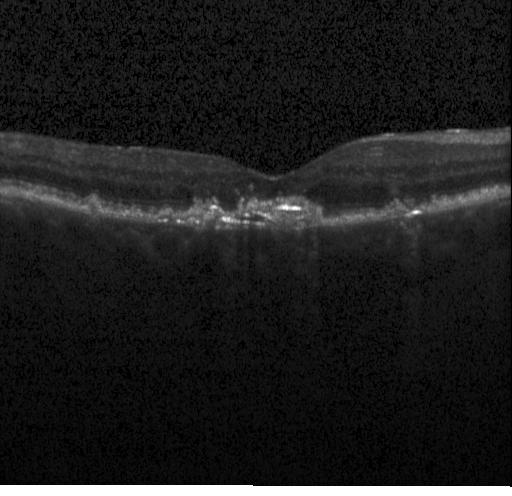

Optical coherence tomography scan
Impression: a choroidal neovascular membrane.